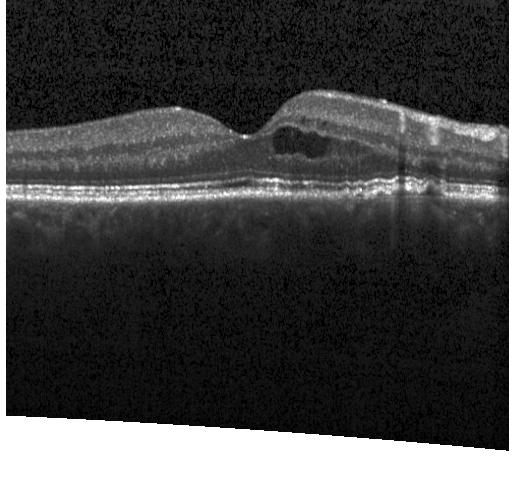
Macular OCT demonstrating CNV.